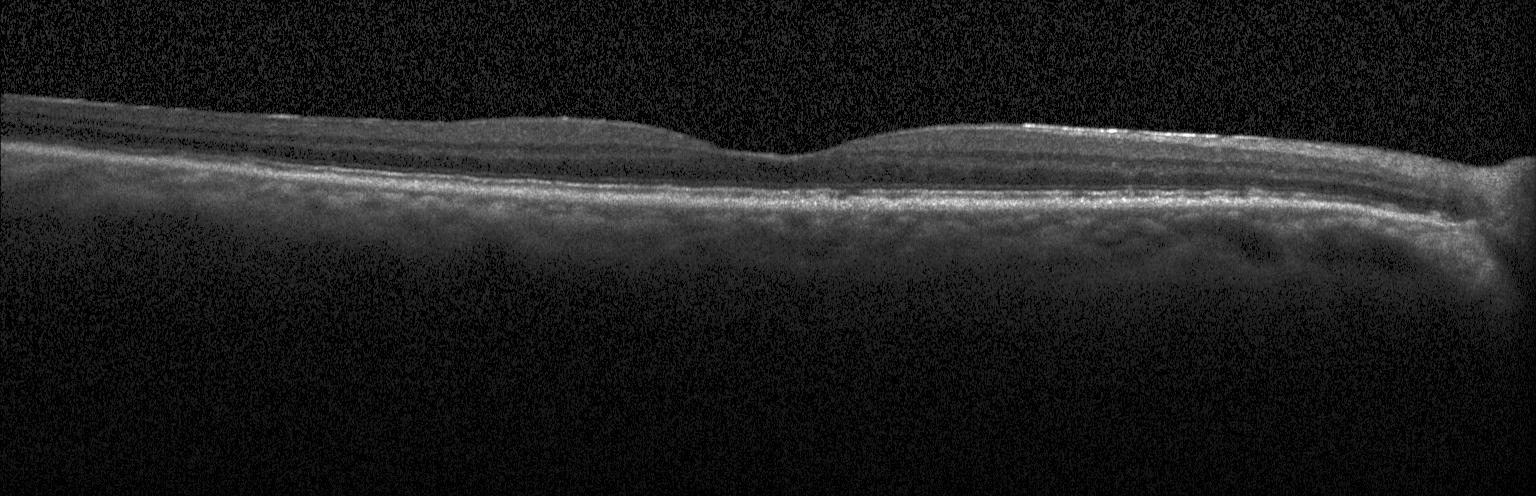

Macular OCT: drusen.